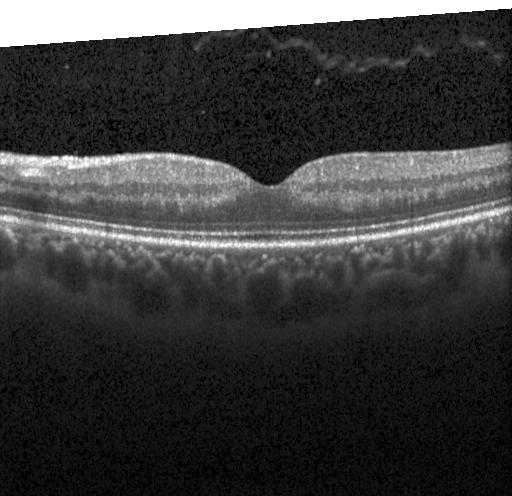 Spectral-domain OCT; OCT line scan; acquired on a Heidelberg Spectralis.
Diagnosis: no choroidal neovascularization, no diabetic macular edema, and no drusen.